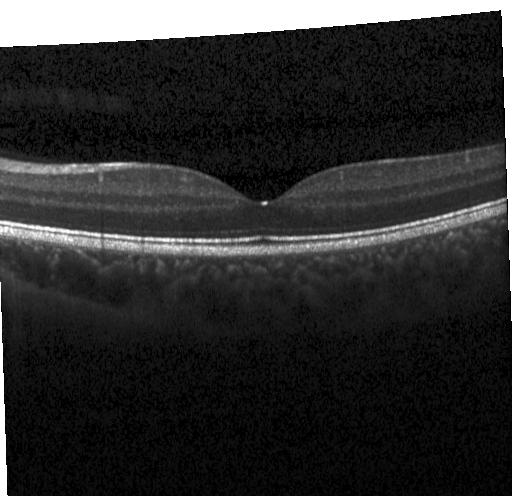

OCT line scan · Heidelberg Spectralis · fovea-centered · spectral-domain OCT.
Diagnosis: neither CNV, DME, nor drusen.